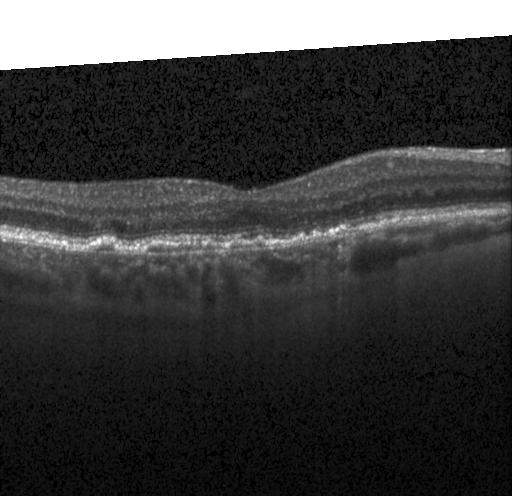
Heidelberg Spectralis OCT system. Spectral-domain optical coherence tomography. Optical coherence tomography scan
Assessment: a choroidal neovascular membrane.